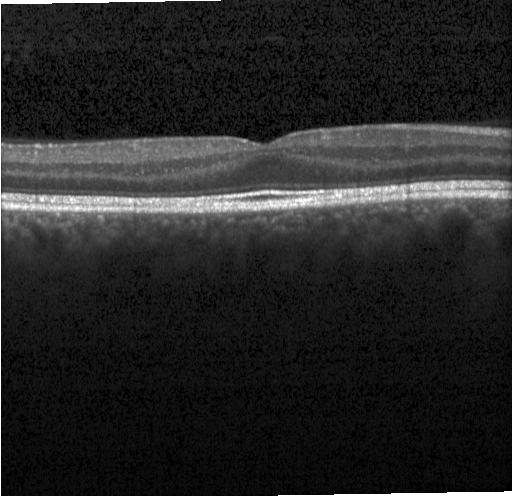
Retinal OCT cross-section showing neither CNV, DME, nor drusen.